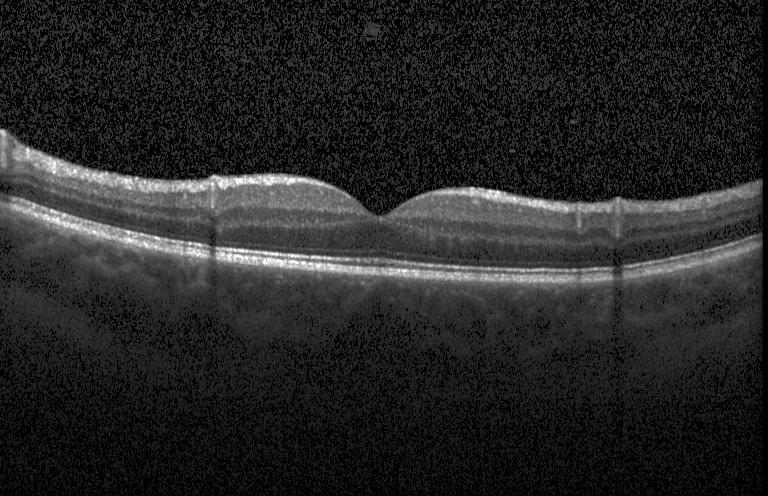

Finding: no evidence of choroidal neovascularization, diabetic macular edema, or drusen.